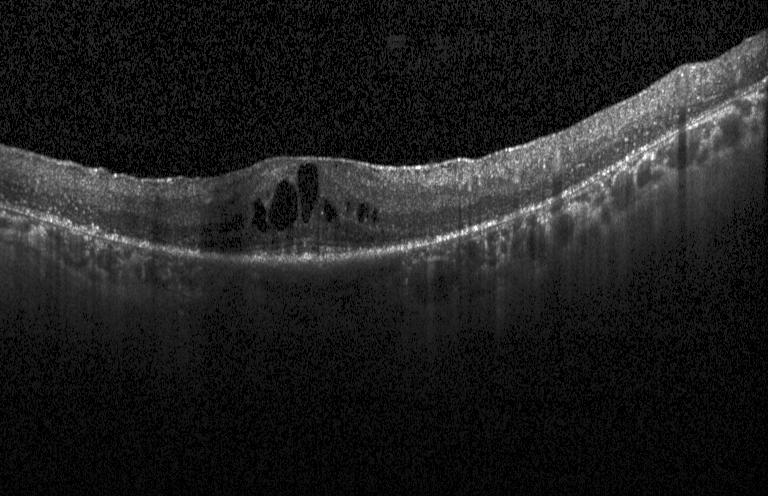 Horizontal scan through the fovea · optical coherence tomography scan. Macular OCT: DME.